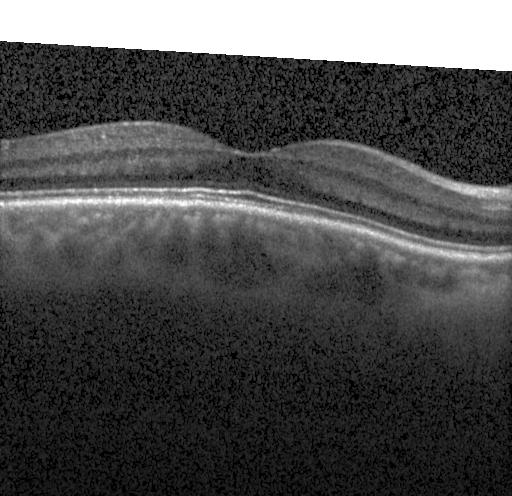
Retinal OCT B-scan — The scan shows neither CNV, DME, nor drusen.